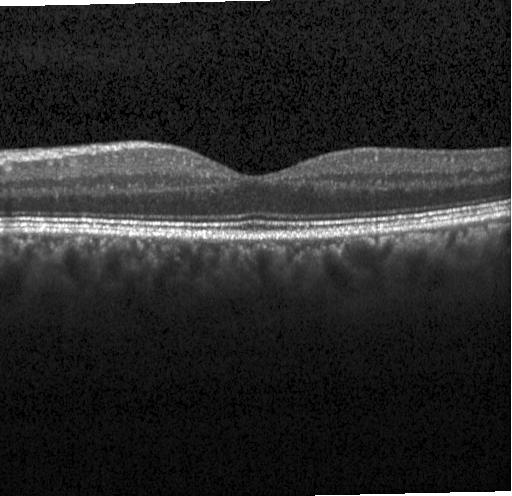 OCT finding: neither choroidal neovascularization, diabetic macular edema, nor drusen.